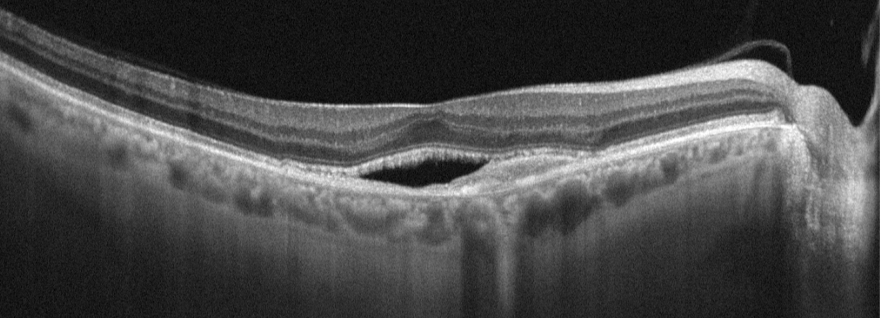 OCT line scan
Assessment: AMD.